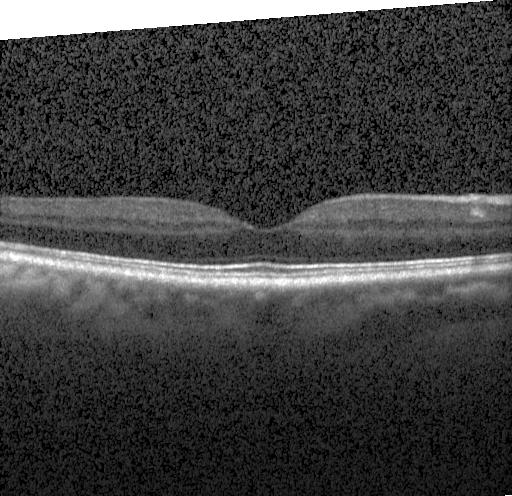

OCT line scan — No evidence of choroidal neovascularization, diabetic macular edema, or drusen.